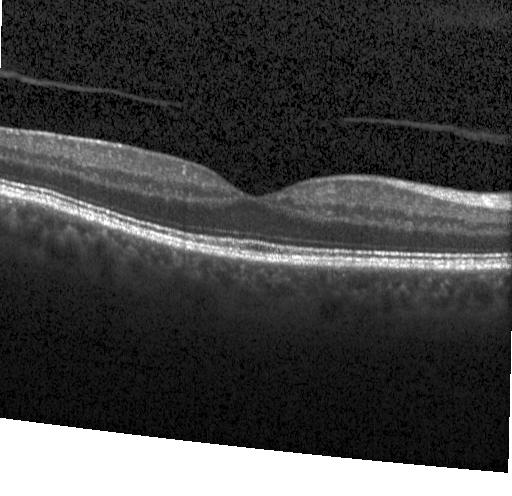

Impression: no choroidal neovascularization, diabetic macular edema, or drusen.